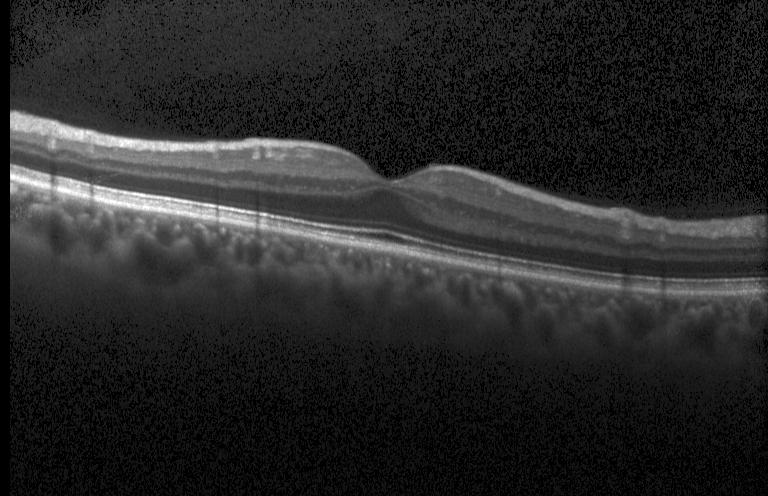 Spectral-domain OCT, through the macula, instrument: Heidelberg Spectralis, retinal OCT B-scan
Finding: no evidence of choroidal neovascularization, diabetic macular edema, or drusen.